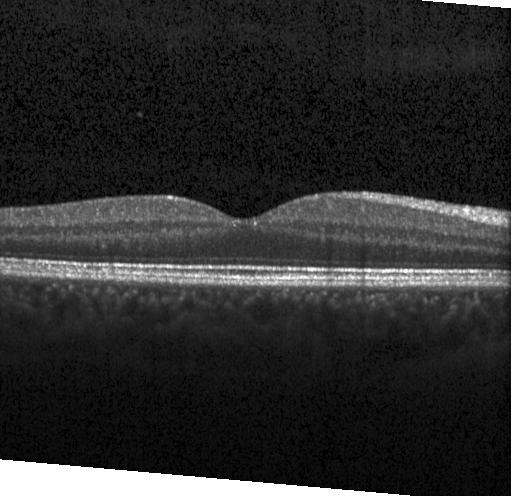
Optical coherence tomography B-scan
Dx: neither CNV, DME, nor drusen.